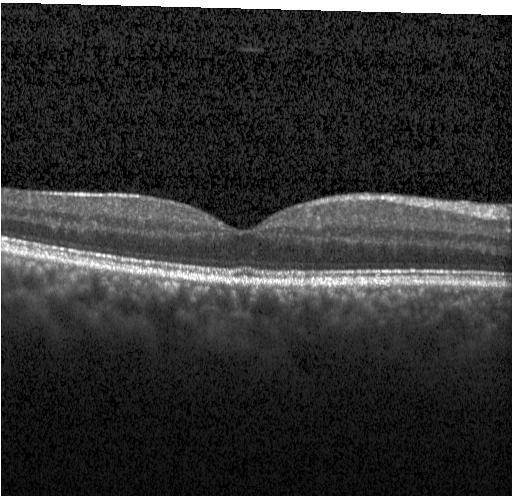

OCT line scan. Assessment: neither CNV, DME, nor drusen.